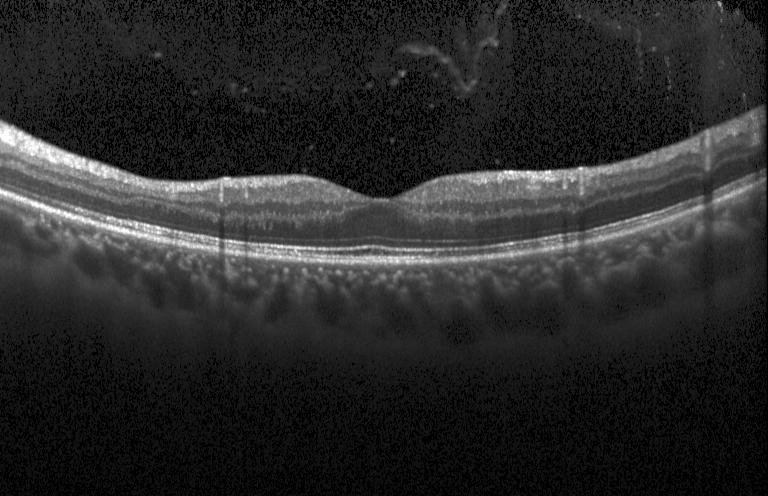 Centered on the fovea. Heidelberg Spectralis OCT system. Retinal OCT B-scan
This B-scan demonstrates neither CNV, DME, nor drusen.